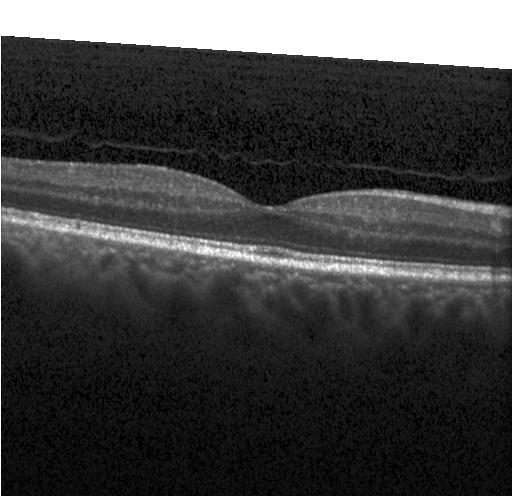
Macular OCT: no choroidal neovascularization, diabetic macular edema, or drusen.